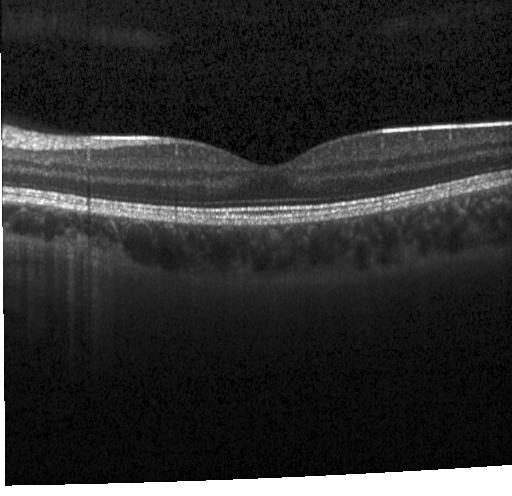

Diagnosis: neither choroidal neovascularization, diabetic macular edema, nor drusen.